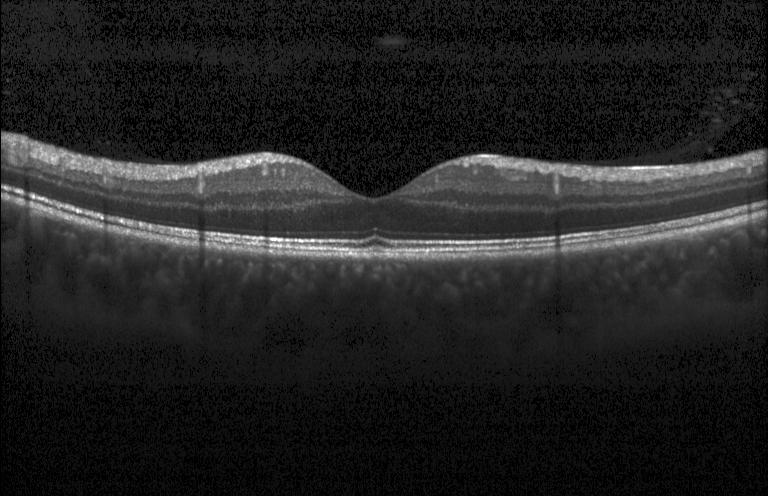
Spectral-domain OCT B-scan: no evidence of CNV, DME, or drusen.